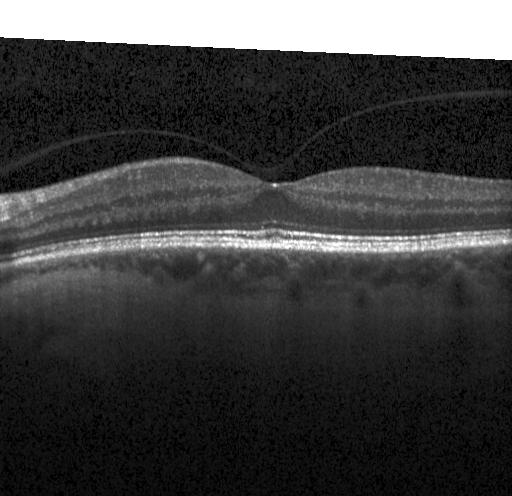

Retinal OCT B-scan, spectral-domain OCT, macular scan.
This B-scan demonstrates no choroidal neovascularization, diabetic macular edema, or drusen.